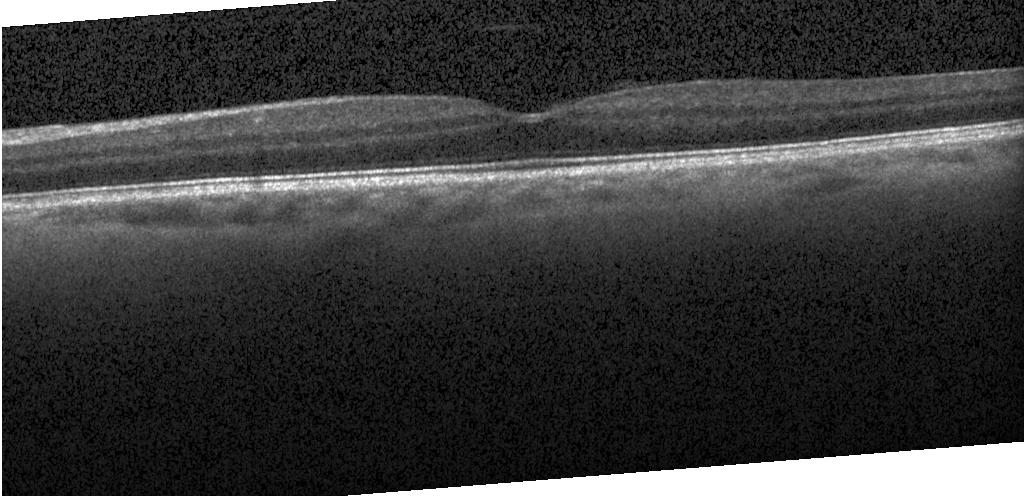

OCT line scan. Instrument: Heidelberg Spectralis. Impression: neither choroidal neovascularization, diabetic macular edema, nor drusen.